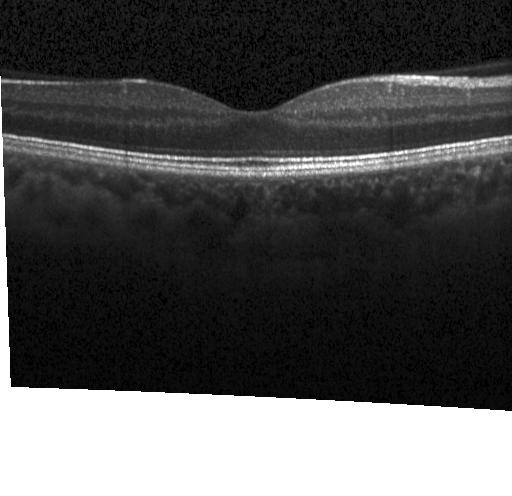
Retinal OCT cross-section. Diagnosis: neither CNV, DME, nor drusen.